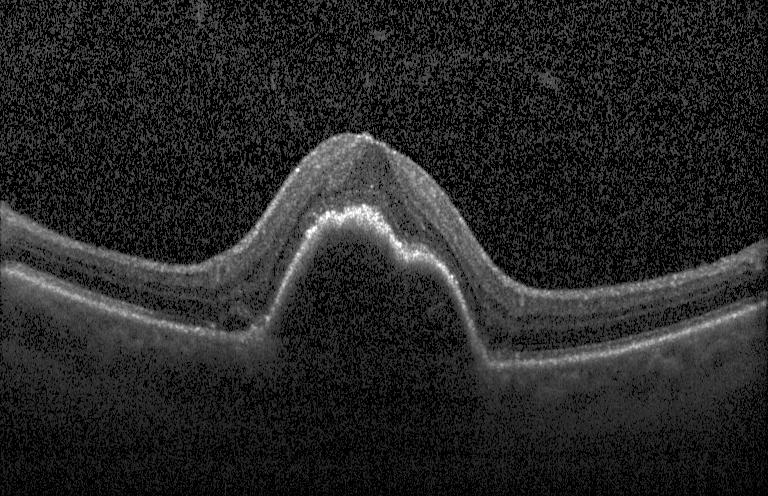

Macular OCT demonstrating choroidal neovascularization (CNV).